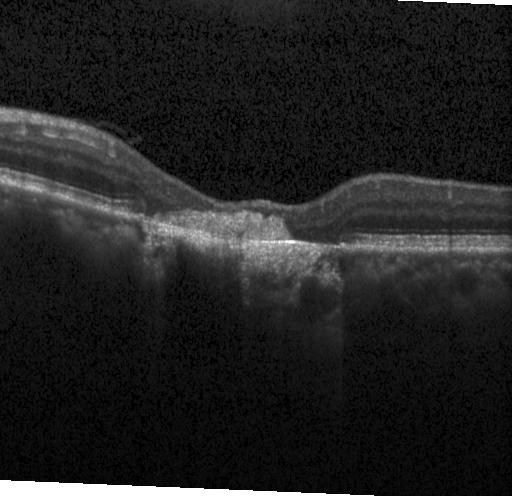
OCT B-scan — Impression: a choroidal neovascular membrane.